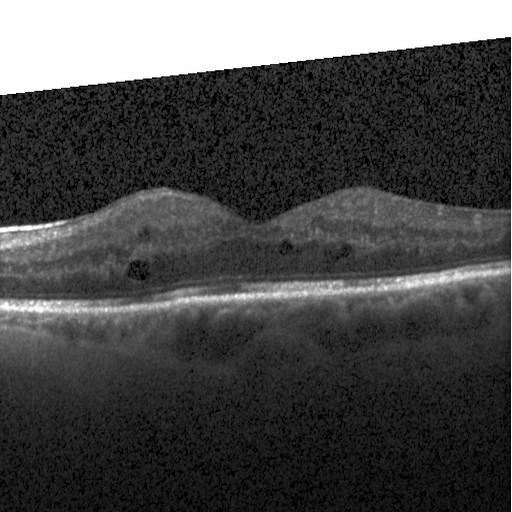 Spectral-domain OCT · optical coherence tomography scan · Heidelberg Spectralis OCT system — Impression: DME.